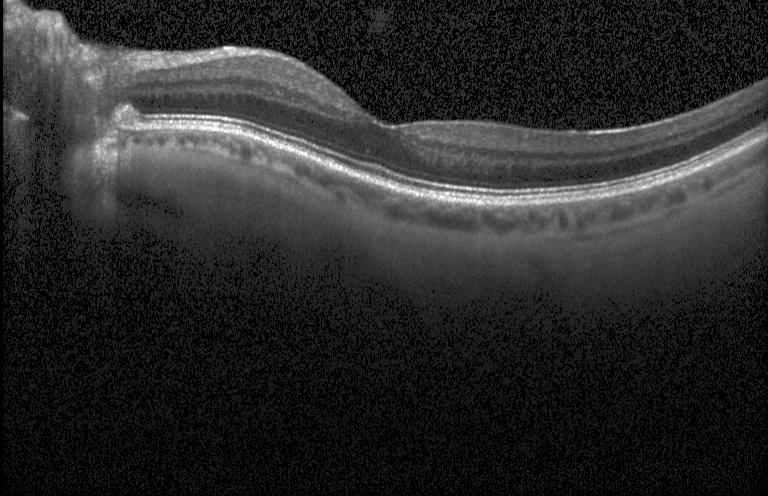

The scan shows sub-RPE drusenoid deposits.